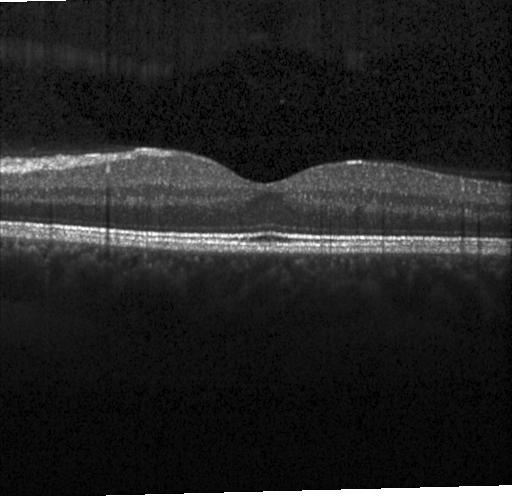
Heidelberg Spectralis · spectral-domain OCT · through the macula · retinal OCT B-scan. Diagnosis: no CNV, no DME, and no drusen.